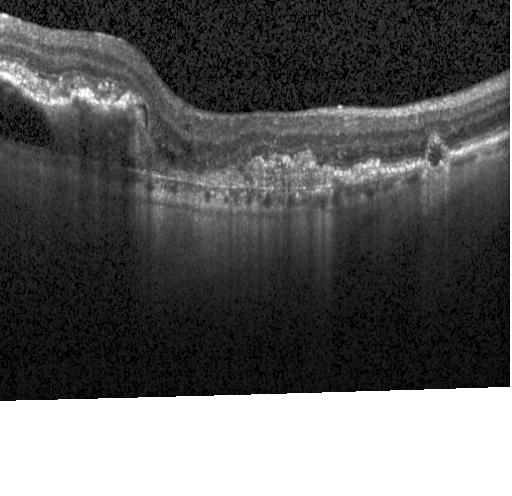 Optical coherence tomography B-scan
Finding: a choroidal neovascular membrane.